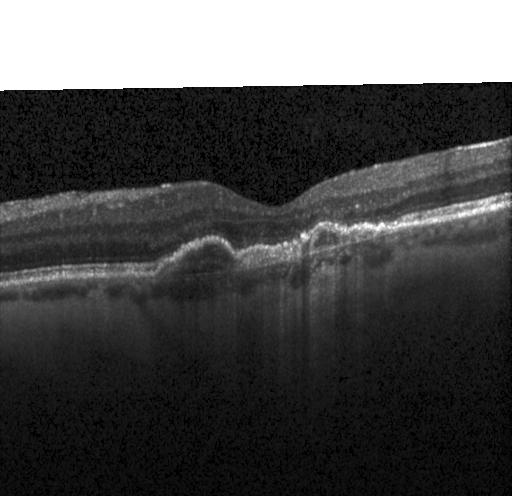 Retinal OCT B-scan · spectral-domain OCT
Finding: choroidal neovascularization (CNV).